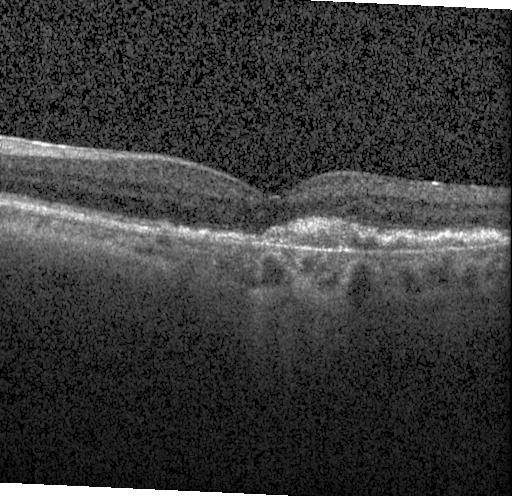 Retinal OCT cross-section, instrument: Heidelberg Spectralis.
Impression: choroidal neovascularization (CNV).